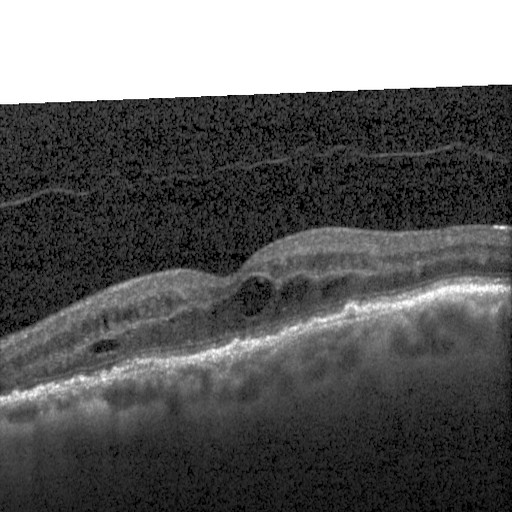

OCT line scan. Dx: diabetic macular edema (DME).